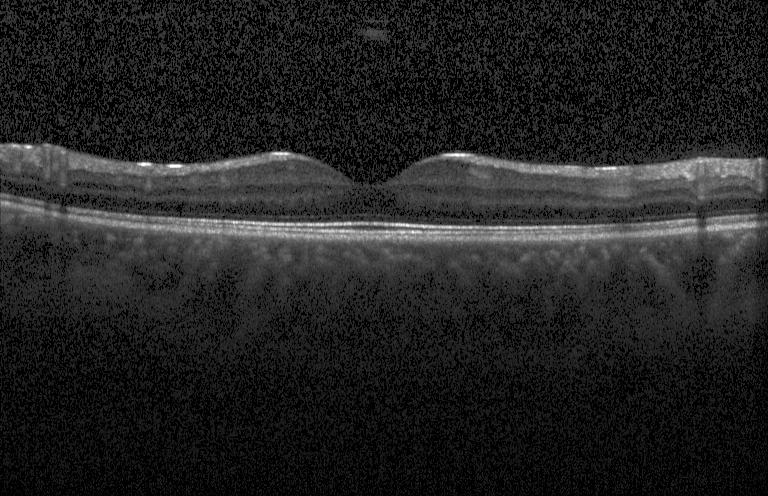

Spectral-domain OCT. Optical coherence tomography scan.
Assessment: no evidence of CNV, DME, or drusen.